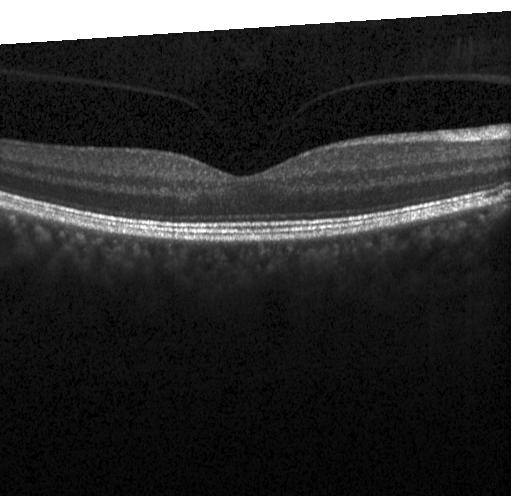
Retinal OCT B-scan. Macular scan — The scan shows no evidence of choroidal neovascularization, diabetic macular edema, or drusen.